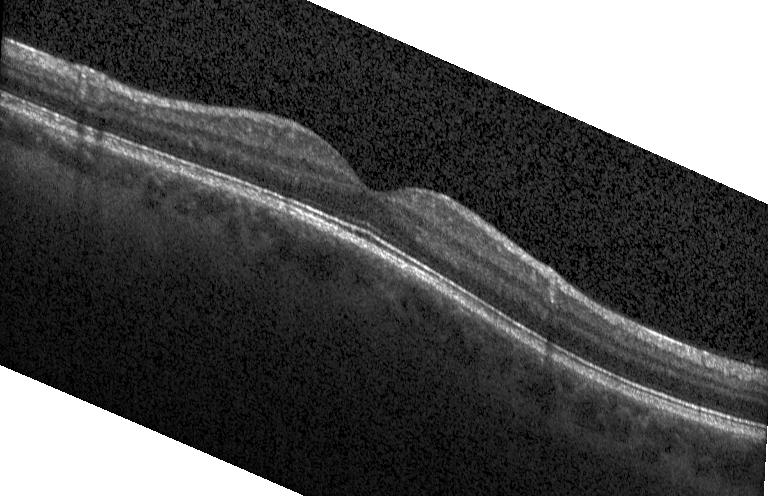

Macular OCT: no choroidal neovascularization, diabetic macular edema, or drusen.